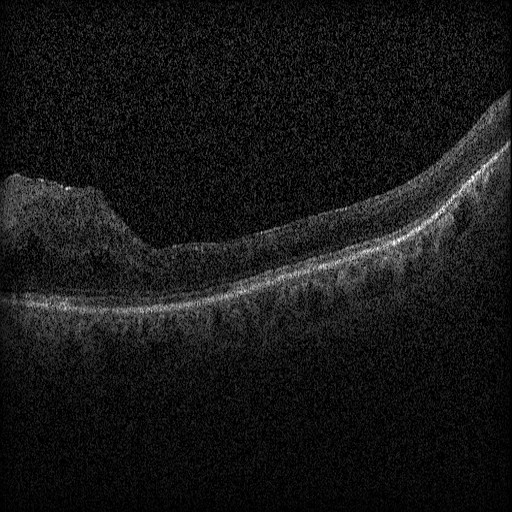 Retinal OCT B-scan · instrument: Heidelberg Spectralis.
The scan shows diabetic macular edema (DME).